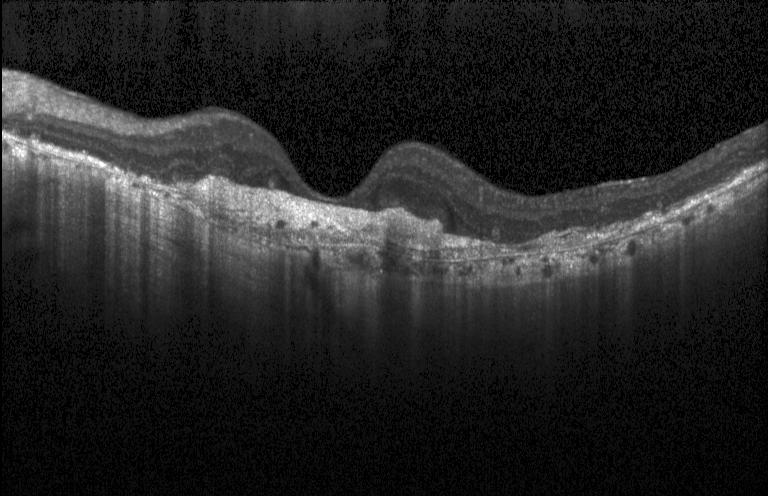

OCT scan showing choroidal neovascularization.